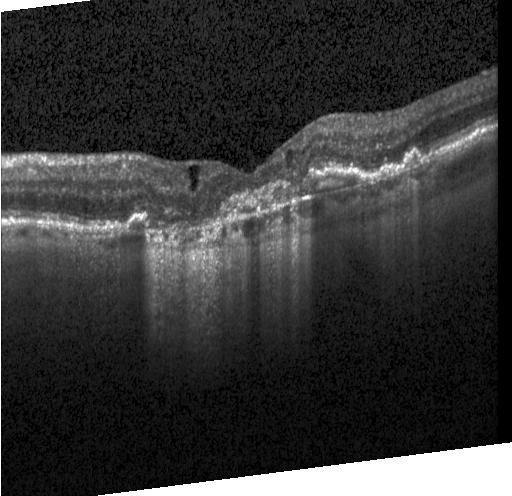
Optical coherence tomography B-scan; instrument: Heidelberg Spectralis
Finding: choroidal neovascularization.